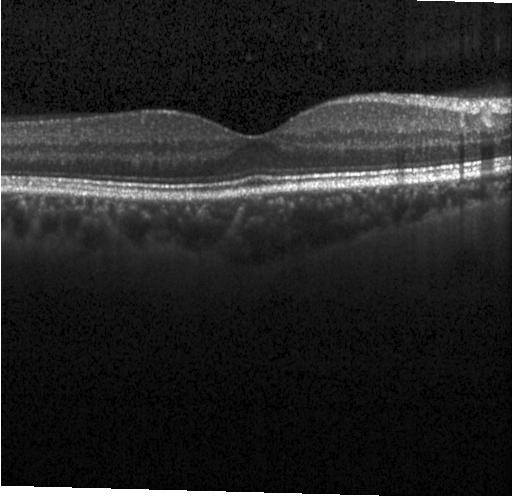

Through the macula · optical coherence tomography B-scan · instrument: Heidelberg Spectralis.
Finding: no evidence of choroidal neovascularization, diabetic macular edema, or drusen.